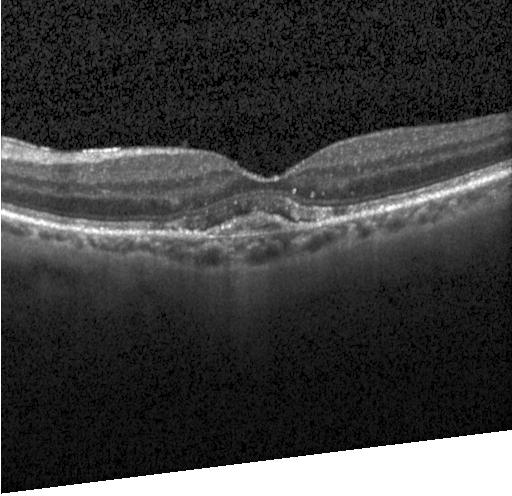
OCT B-scan, SD-OCT.
Macular OCT: choroidal neovascularization (CNV).